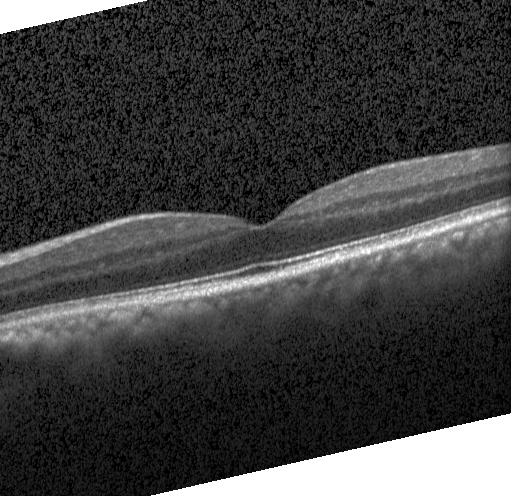

Spectral-domain OCT B-scan: no choroidal neovascularization, diabetic macular edema, or drusen.